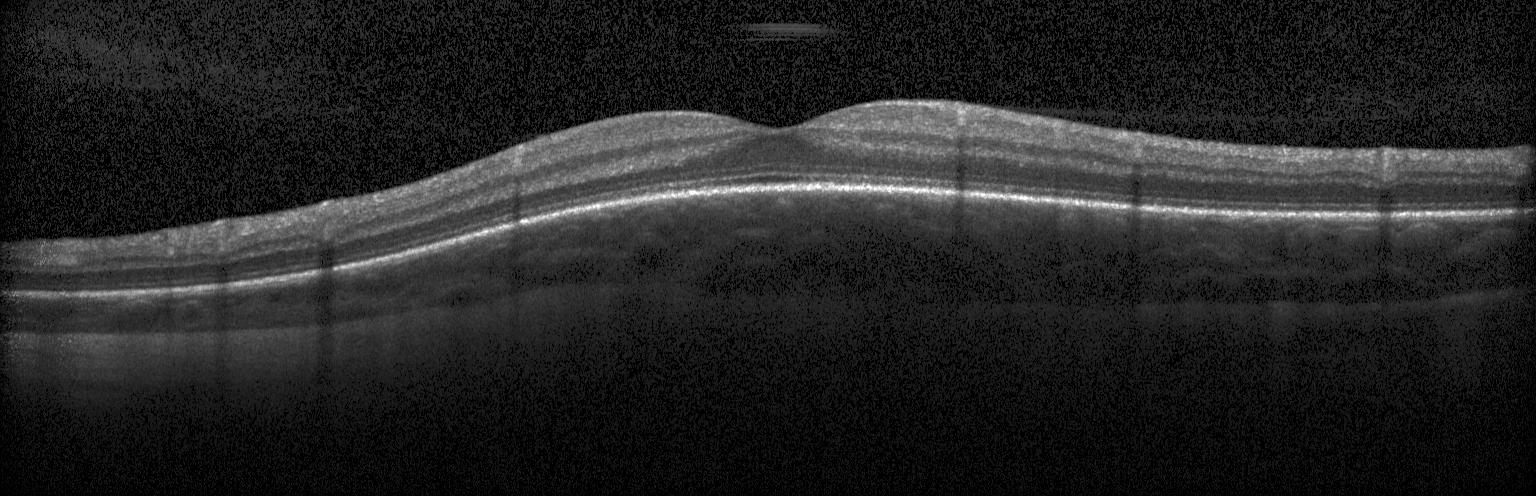

Spectral-domain optical coherence tomography, centered on the fovea, acquired on a Heidelberg Spectralis, retinal OCT cross-section. Macular OCT: neither choroidal neovascularization, diabetic macular edema, nor drusen.